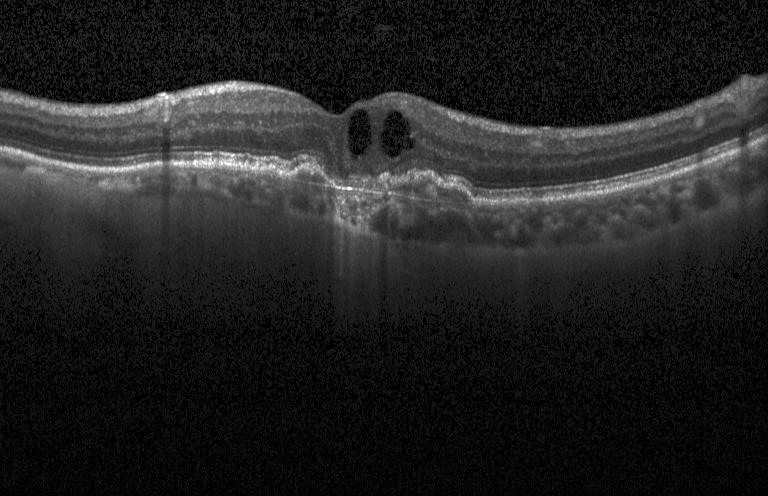 Spectral-domain optical coherence tomography, centered on the fovea, optical coherence tomography scan, Heidelberg Spectralis — CNV.